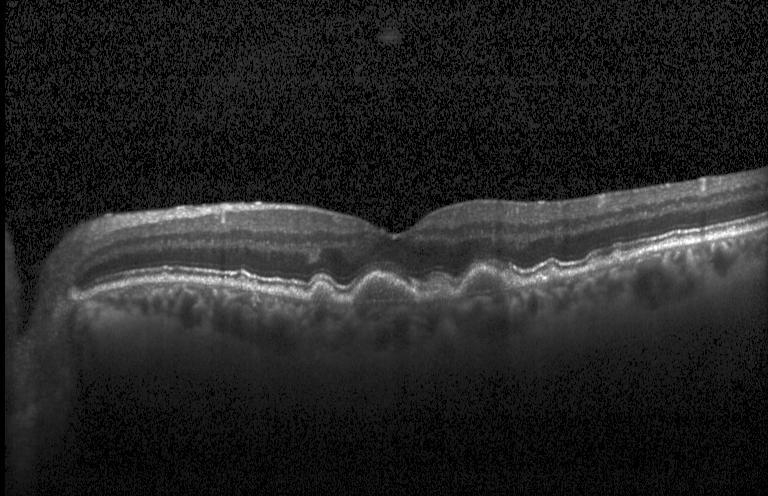 Finding: multiple drusen.